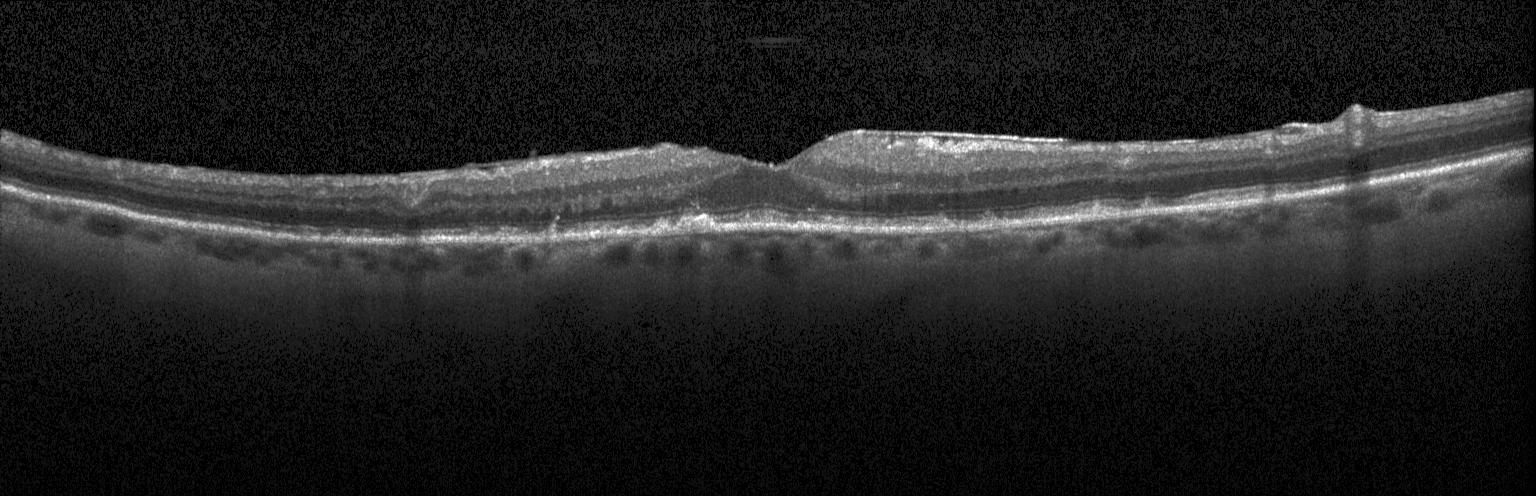

Diagnosis: multiple drusen.